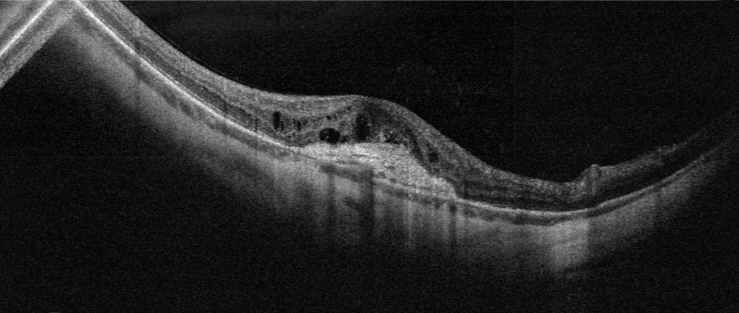 Macular scan. Optical coherence tomography B-scan.
Macular OCT: age-related macular degeneration (AMD).